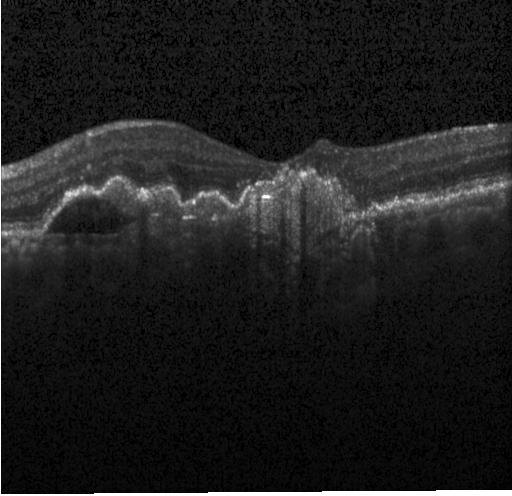

Dx: a choroidal neovascular membrane.